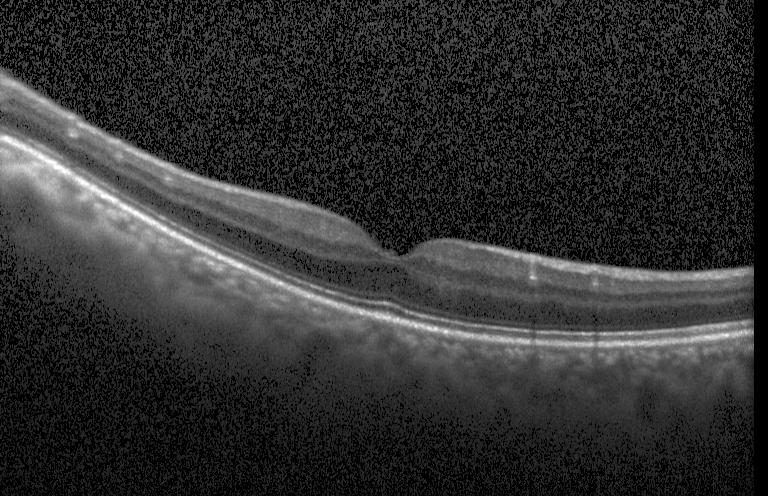
OCT B-scan showing neither choroidal neovascularization, diabetic macular edema, nor drusen.